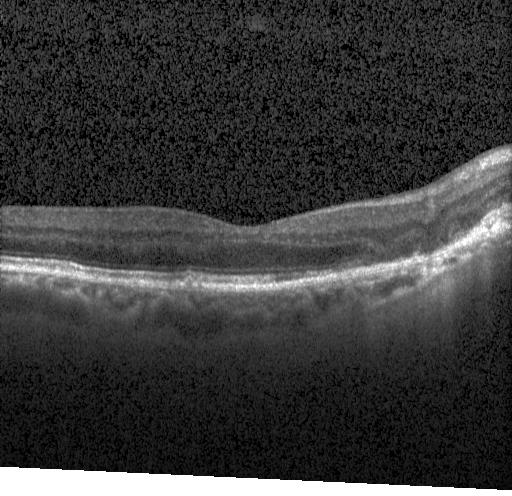

Diagnosis: a choroidal neovascular membrane.